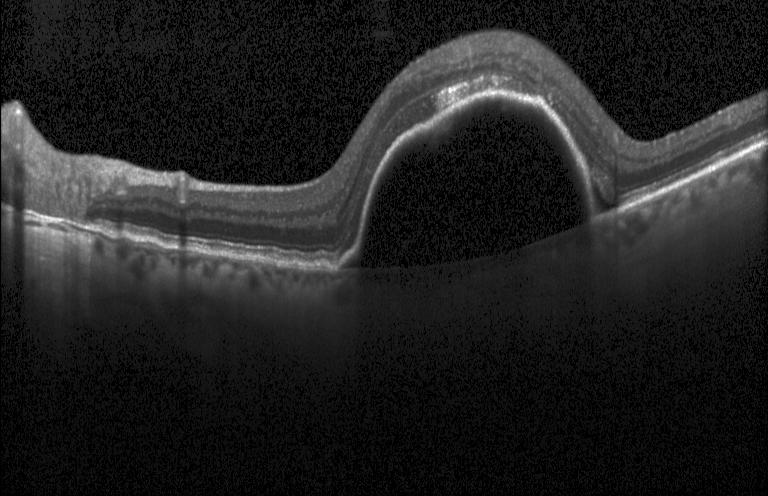
Acquired on a Heidelberg Spectralis, retinal OCT cross-section, through the macula. Choroidal neovascularization.